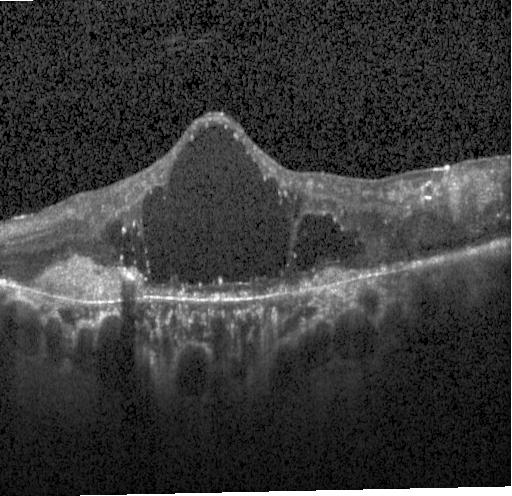

OCT finding: a choroidal neovascular membrane.